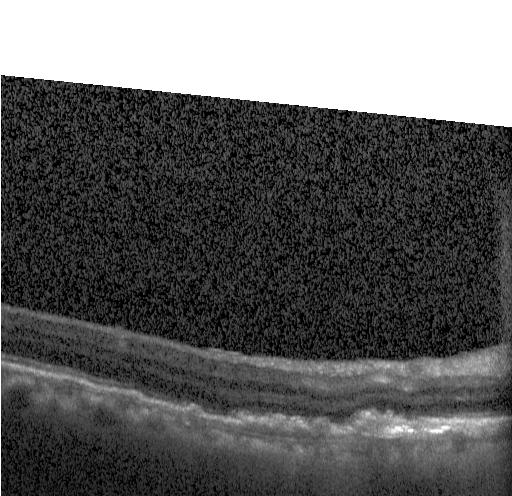
Optical coherence tomography B-scan.
Finding: a choroidal neovascular membrane.